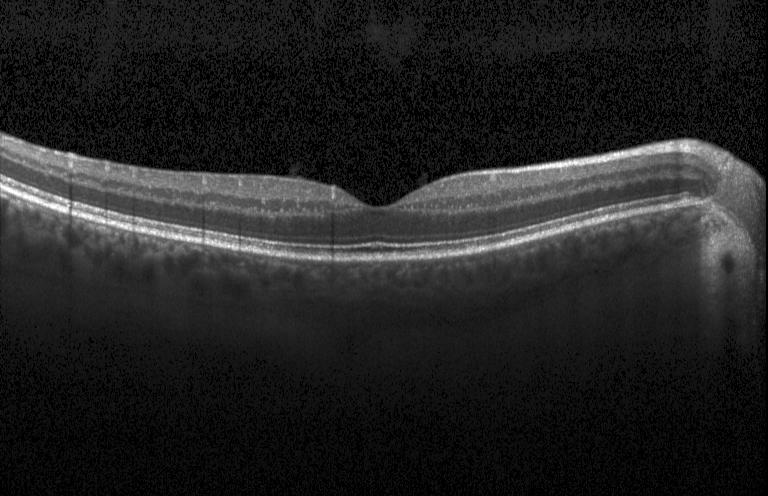 Neither choroidal neovascularization, diabetic macular edema, nor drusen.